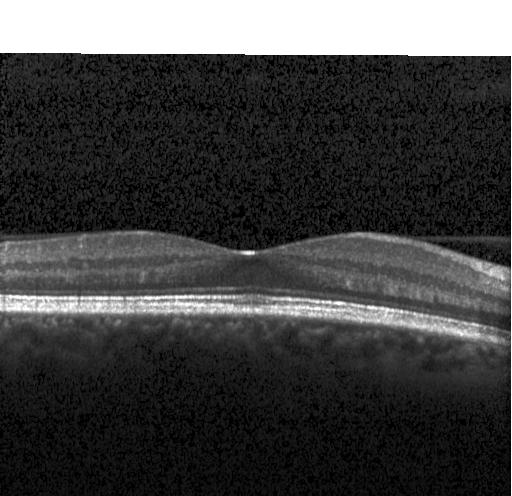
Macular OCT: no evidence of CNV, DME, or drusen.